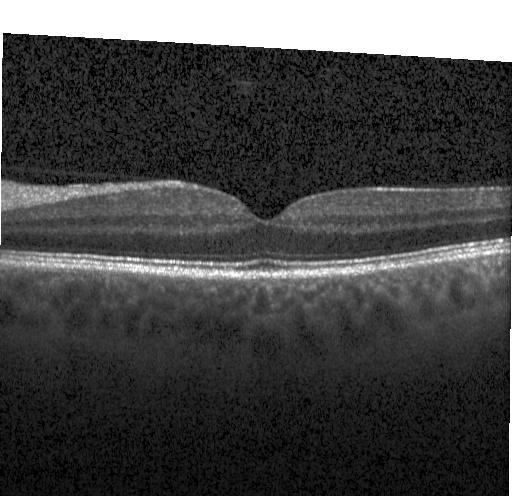
OCT B-scan. Diagnosis: no choroidal neovascularization, diabetic macular edema, or drusen.